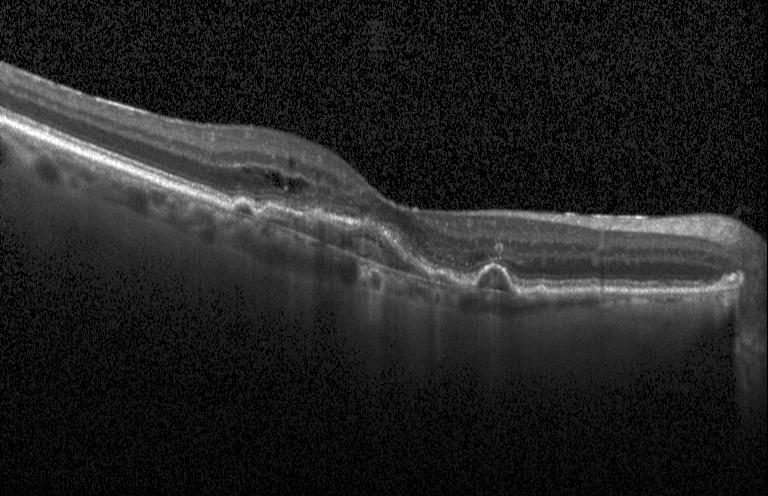
Spectral-domain OCT B-scan: CNV.